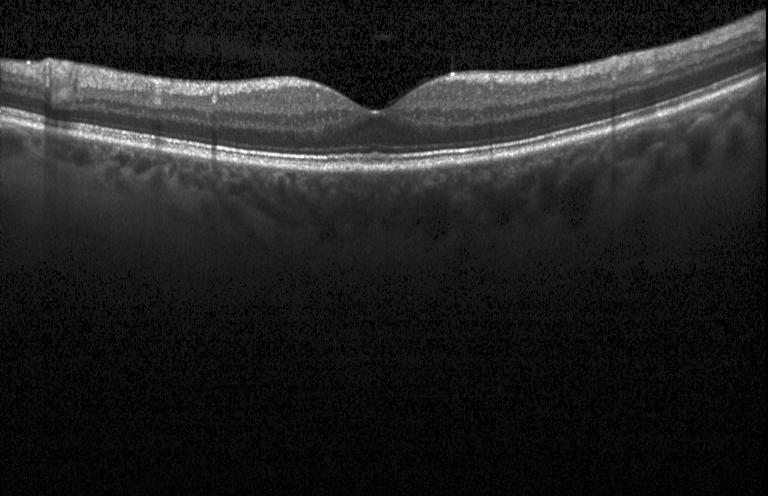
Impression: no CNV, DME, or drusen.